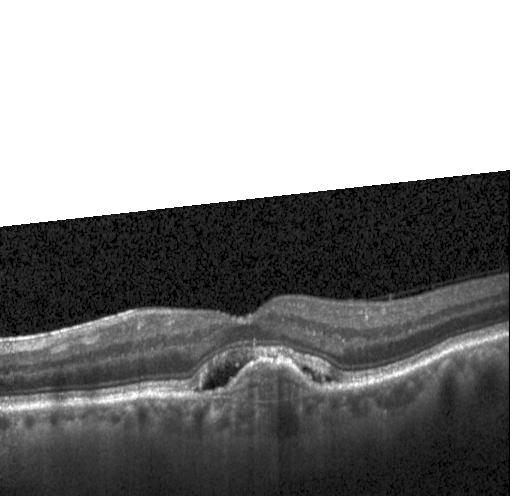 OCT B-scan, acquired on a Heidelberg Spectralis, macular scan, spectral-domain OCT
Macular OCT: a choroidal neovascular membrane.